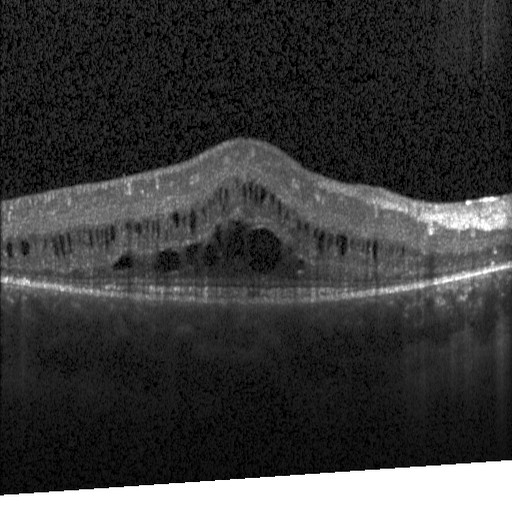 Retinal OCT cross-section — Macular OCT: DME.